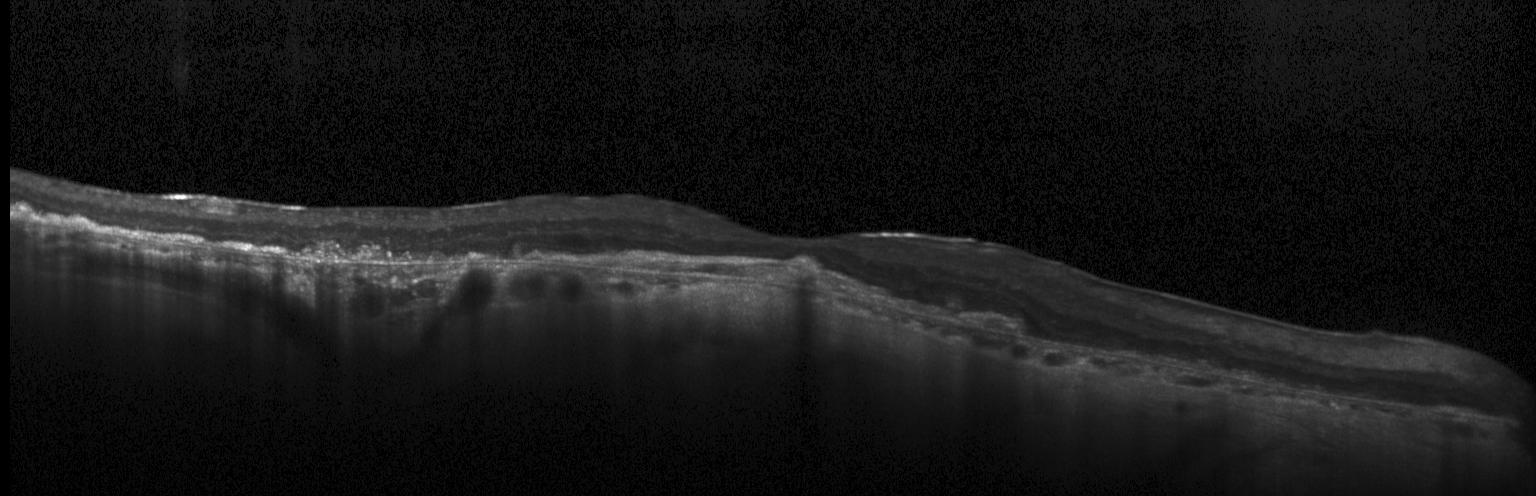

Finding: CNV.